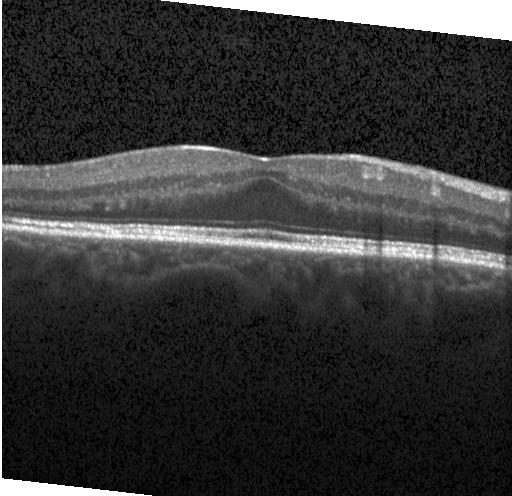
Heidelberg Spectralis, through the macula, optical coherence tomography scan
Impression: no evidence of CNV, DME, or drusen.